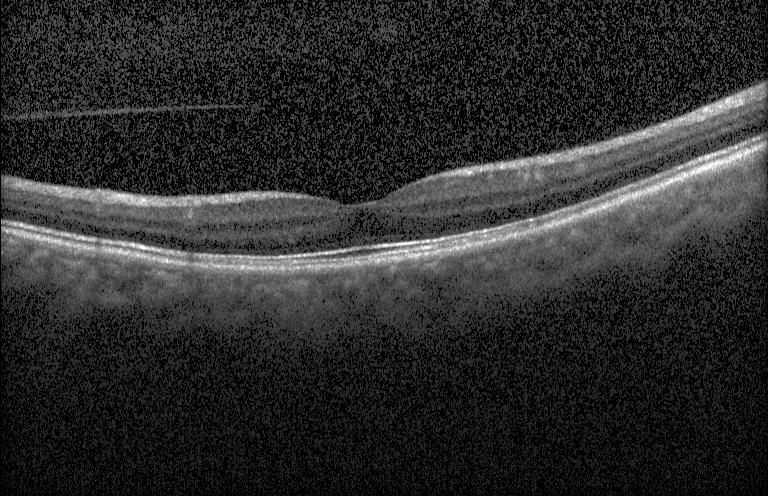

OCT scan showing no evidence of choroidal neovascularization, diabetic macular edema, or drusen.